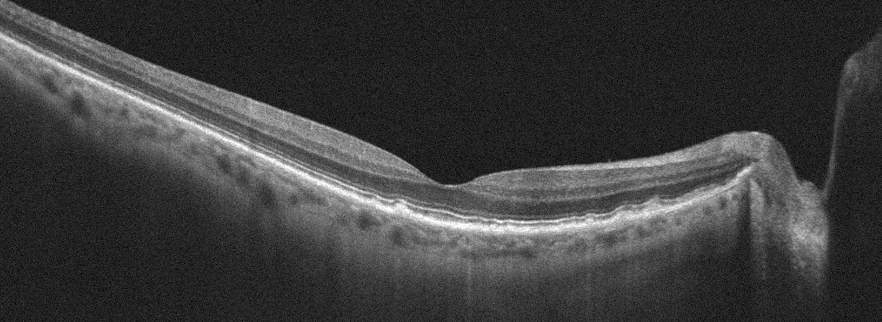 Retinal OCT cross-section · OD — Finding: age-related macular degeneration.